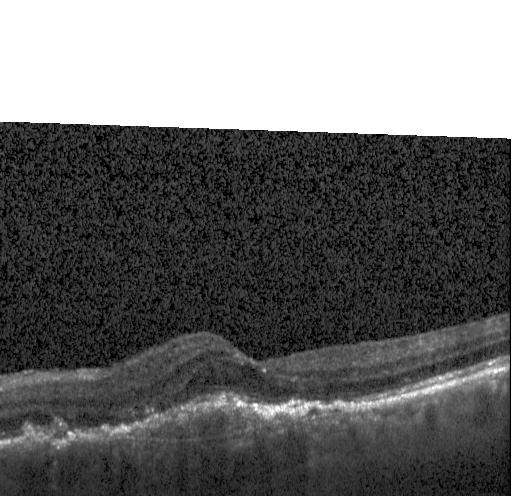 Diagnosis: a choroidal neovascular membrane.